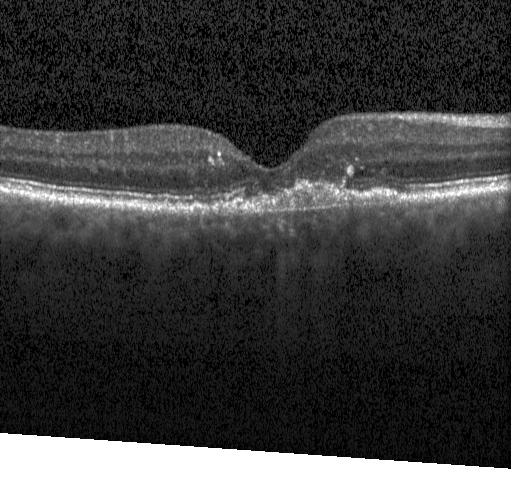 Impression: a choroidal neovascular membrane.